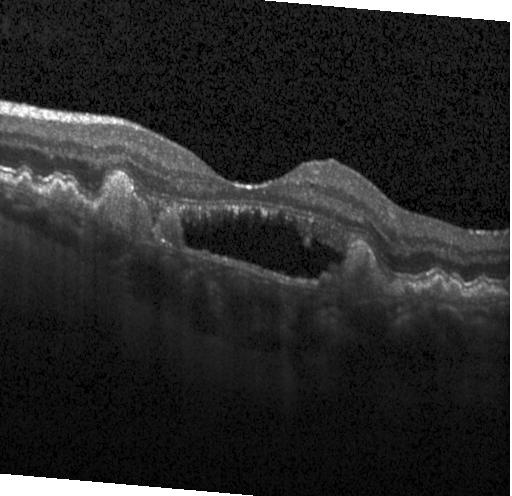
Instrument: Heidelberg Spectralis, spectral-domain OCT, optical coherence tomography scan, centered on the fovea.
Diagnosis: CNV.